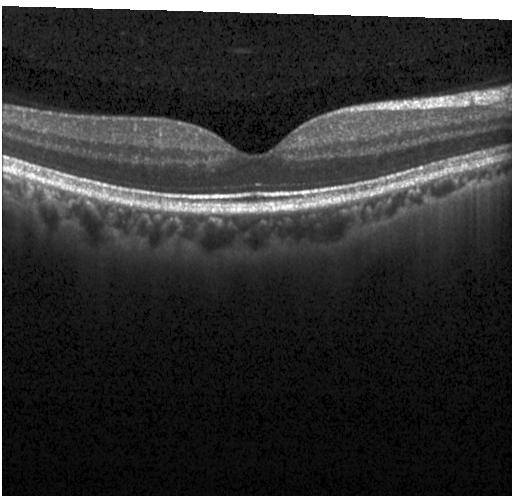

Assessment: no evidence of choroidal neovascularization, diabetic macular edema, or drusen.